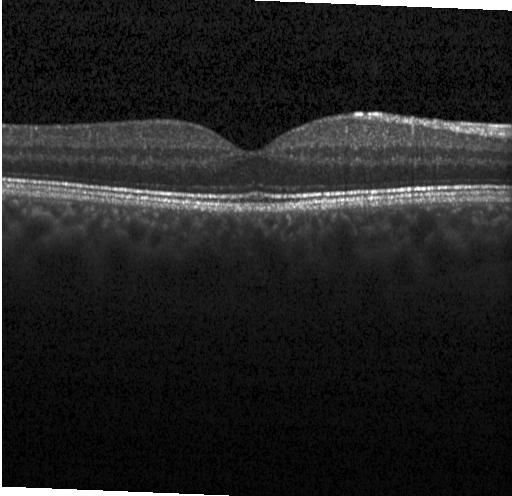

Impression: neither choroidal neovascularization, diabetic macular edema, nor drusen.